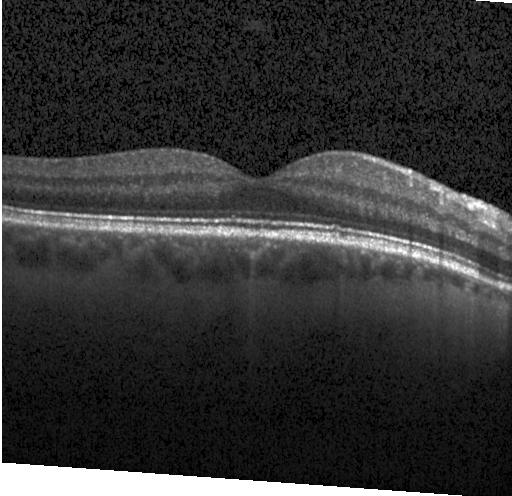

Centered on the fovea · optical coherence tomography B-scan · acquired on a Heidelberg Spectralis. Finding: neither choroidal neovascularization, diabetic macular edema, nor drusen.